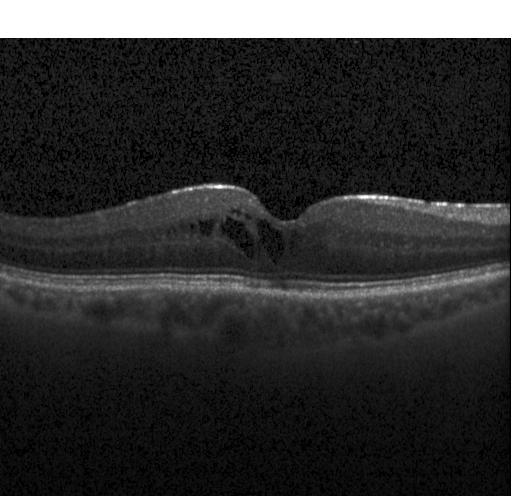
Optical coherence tomography scan.
OCT finding: diabetic macular edema (DME).